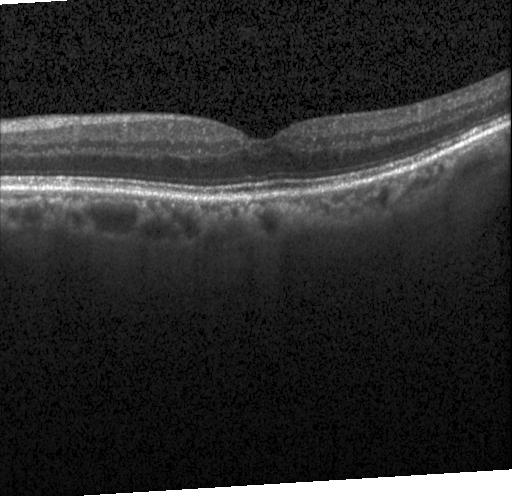 Retinal OCT B-scan. Centered on the fovea. SD-OCT
Diagnosis: no CNV, DME, or drusen.